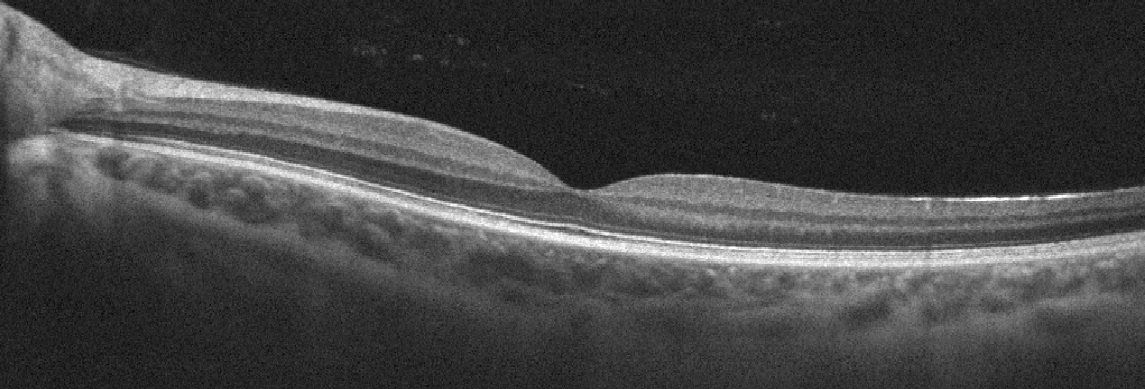
OCT B-scan showing no AMD, DME, ERM, RAO, RVO, or VID.